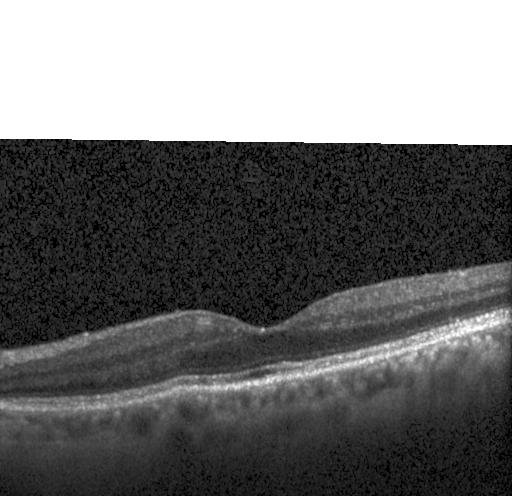
Dx: neither choroidal neovascularization, diabetic macular edema, nor drusen.